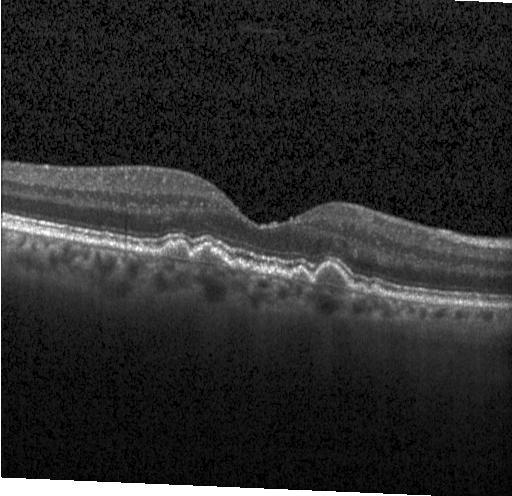
Retinal OCT cross-section
Assessment: drusen.